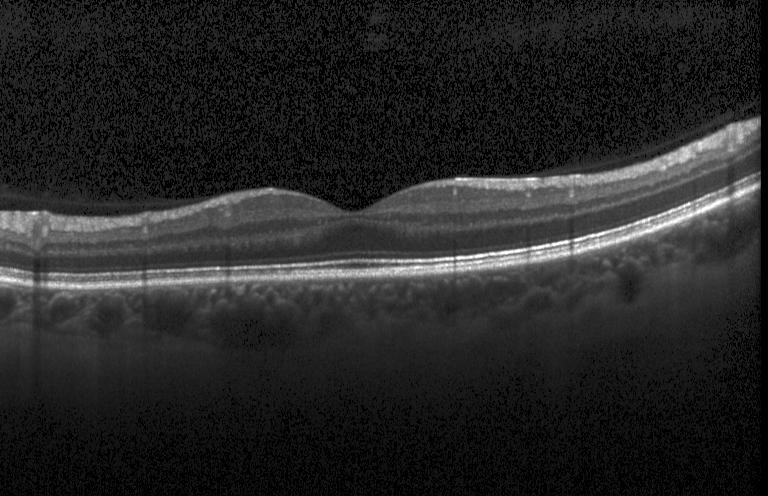

Spectral-domain optical coherence tomography, horizontal scan through the fovea, retinal OCT B-scan
The scan shows no evidence of CNV, DME, or drusen.